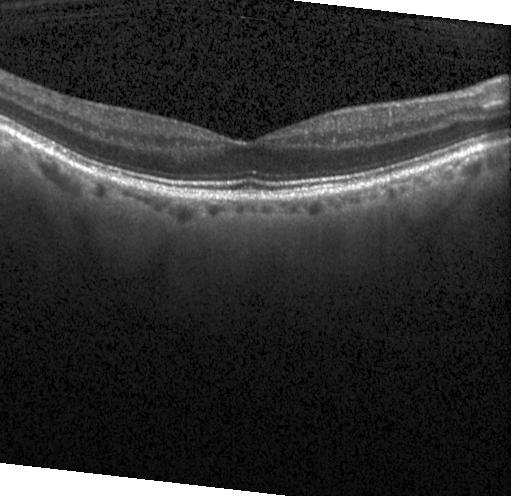

Centered on the fovea, OCT B-scan.
Diagnosis: no choroidal neovascularization, no diabetic macular edema, and no drusen.